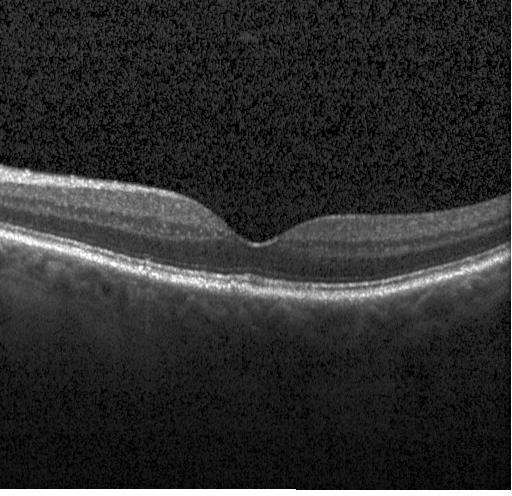
OCT scan showing neither choroidal neovascularization, diabetic macular edema, nor drusen.